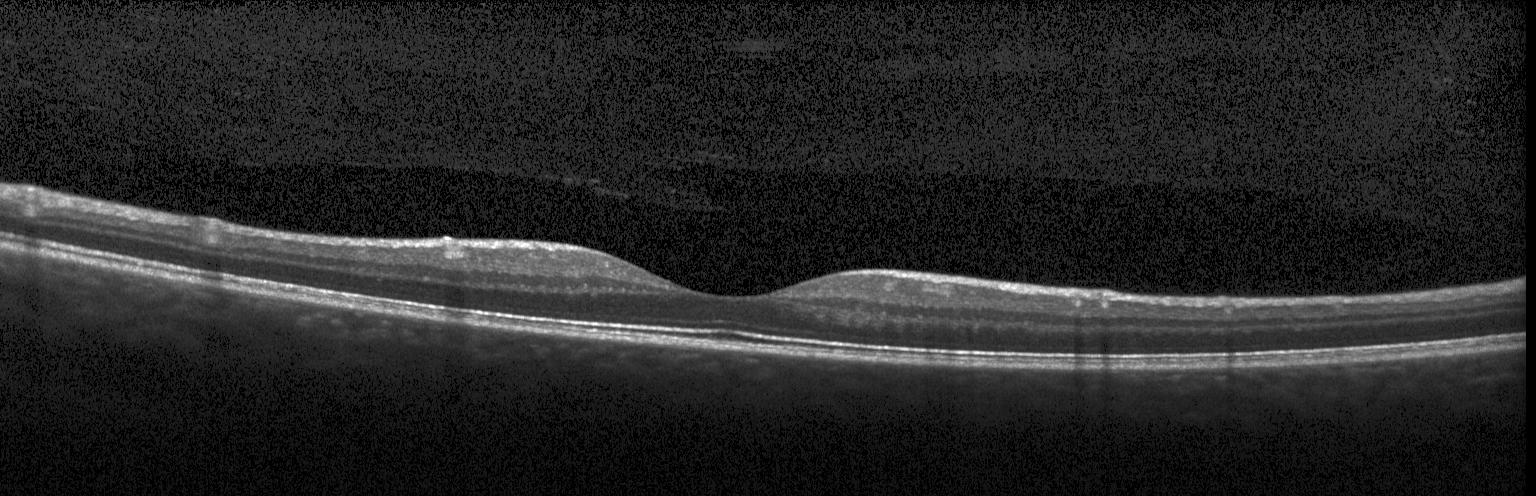
Instrument: Heidelberg Spectralis. OCT B-scan. Fovea-centered. SD-OCT — Dx: no CNV, DME, or drusen.